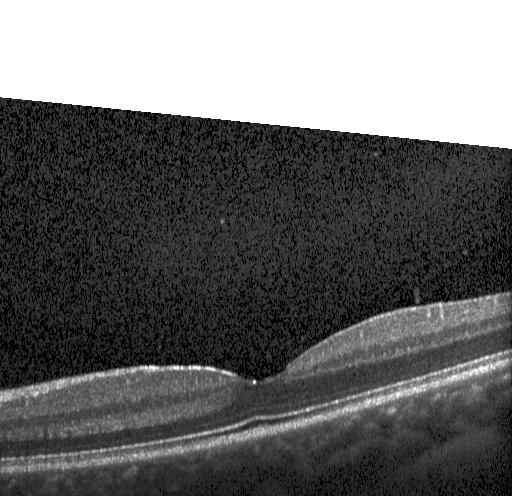
The scan shows neither choroidal neovascularization, diabetic macular edema, nor drusen.